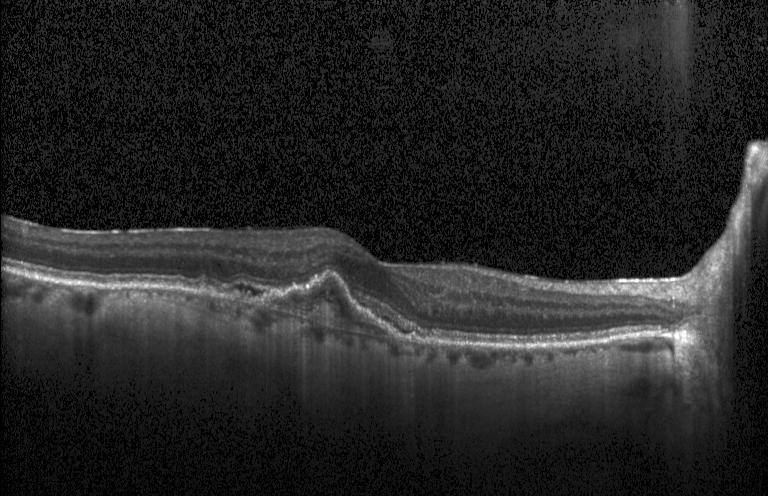
Spectral-domain optical coherence tomography. Acquired on a Heidelberg Spectralis. Optical coherence tomography B-scan
Diagnosis: choroidal neovascularization.